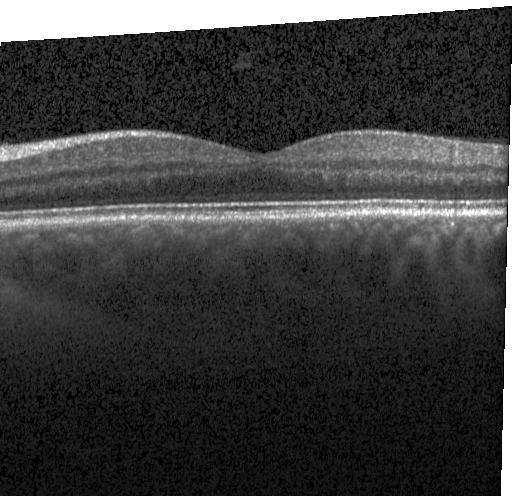
OCT finding: neither CNV, DME, nor drusen.